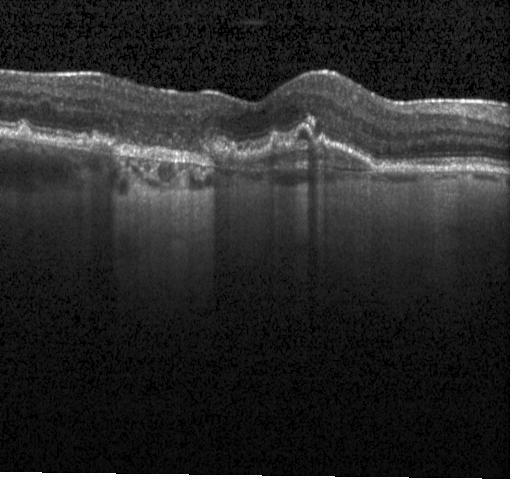

Spectral-domain OCT B-scan: CNV.